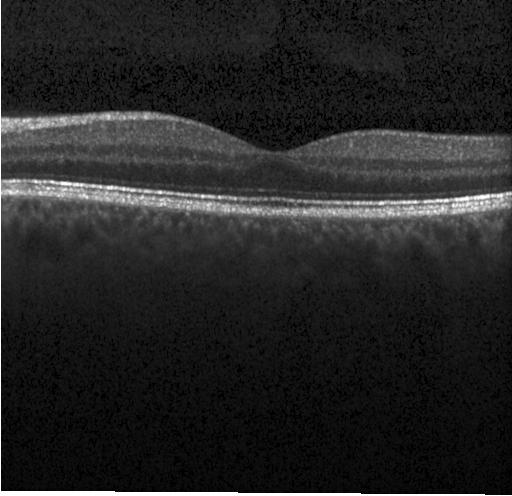

Dx: no evidence of choroidal neovascularization, diabetic macular edema, or drusen.